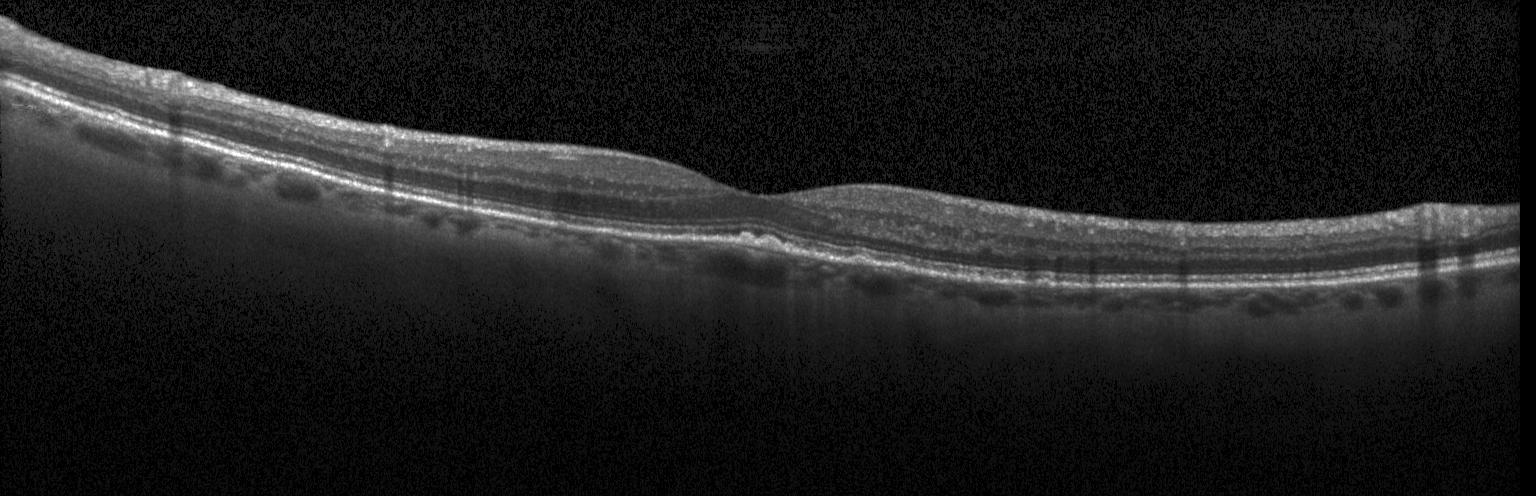

OCT B-scan.
Finding: sub-RPE drusenoid deposits.